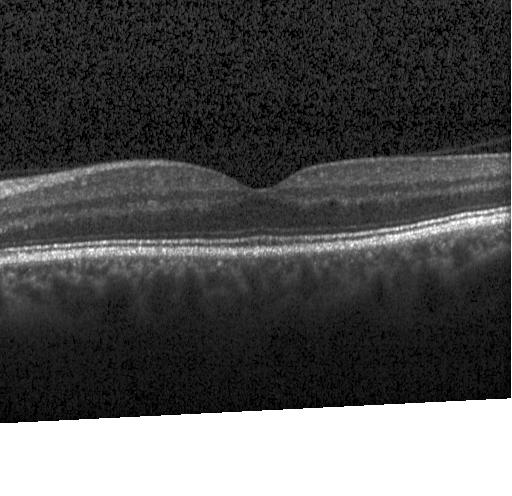

SD-OCT; instrument: Heidelberg Spectralis; macular scan; retinal OCT cross-section.
The scan shows no choroidal neovascularization, diabetic macular edema, or drusen.